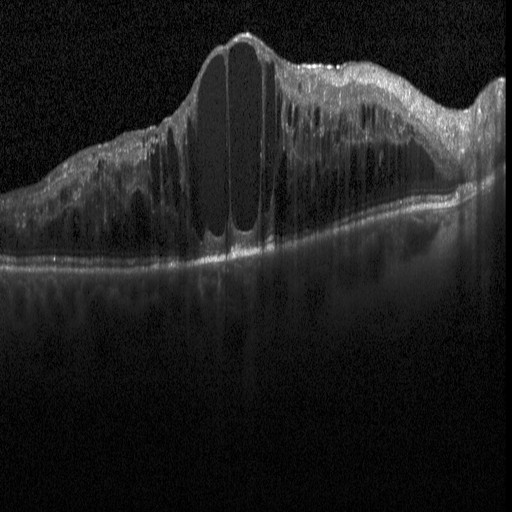

Diagnosis: diabetic macular edema.